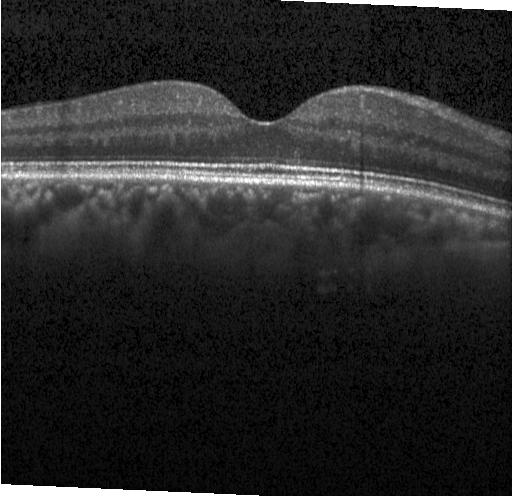 No CNV, no DME, and no drusen.